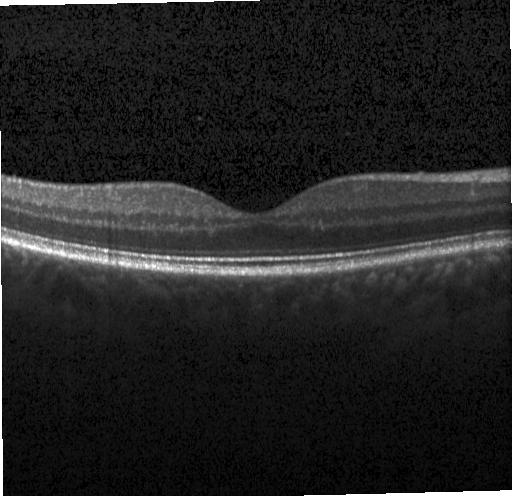 Retinal OCT cross-section. SD-OCT. Acquired on a Heidelberg Spectralis. Through the macula. Macular OCT: no choroidal neovascularization, diabetic macular edema, or drusen.